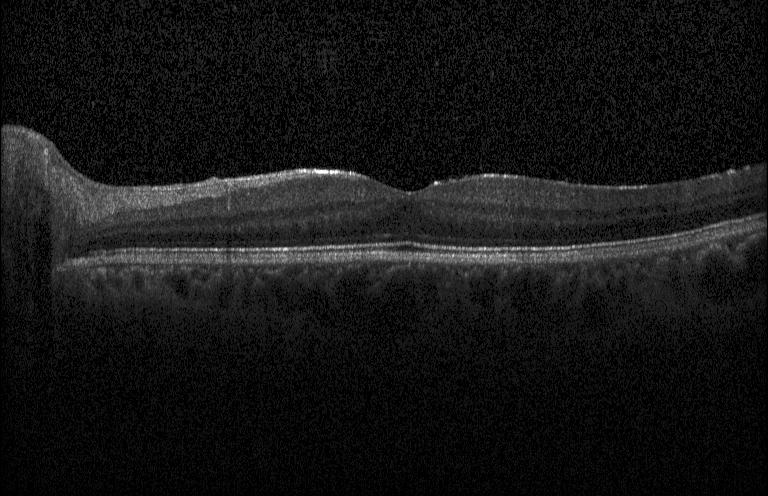
SD-OCT, optical coherence tomography B-scan, centered on the fovea, acquired on a Heidelberg Spectralis — Assessment: no choroidal neovascularization, no diabetic macular edema, and no drusen.